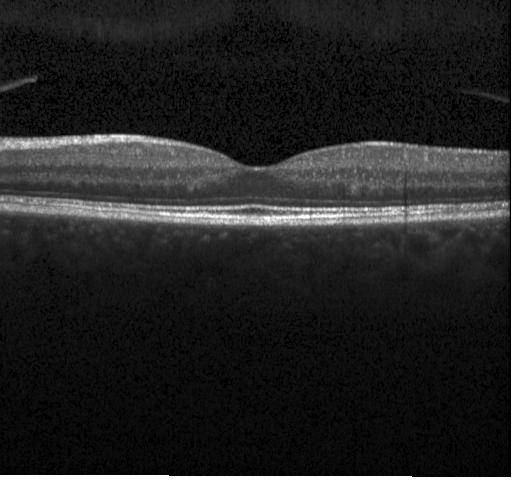
Heidelberg Spectralis OCT system; retinal OCT cross-section.
Impression: no CNV, no DME, and no drusen.